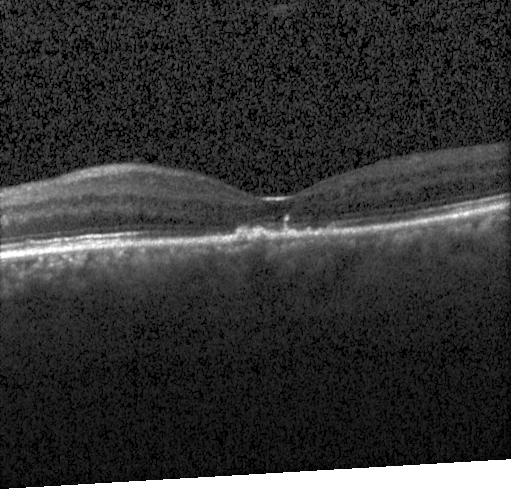
Spectral-domain OCT B-scan: sub-RPE drusenoid deposits.